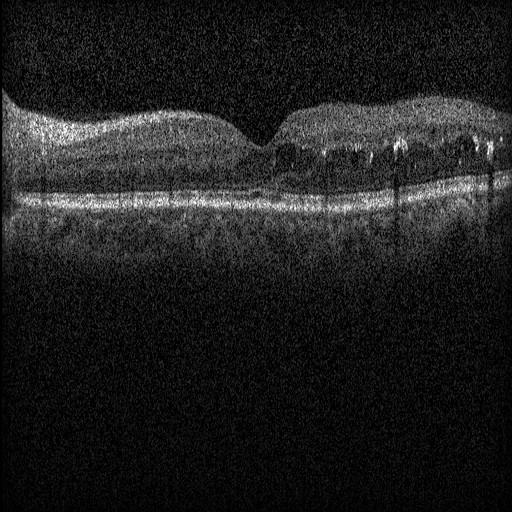

Diagnosis: diabetic macular edema (DME).